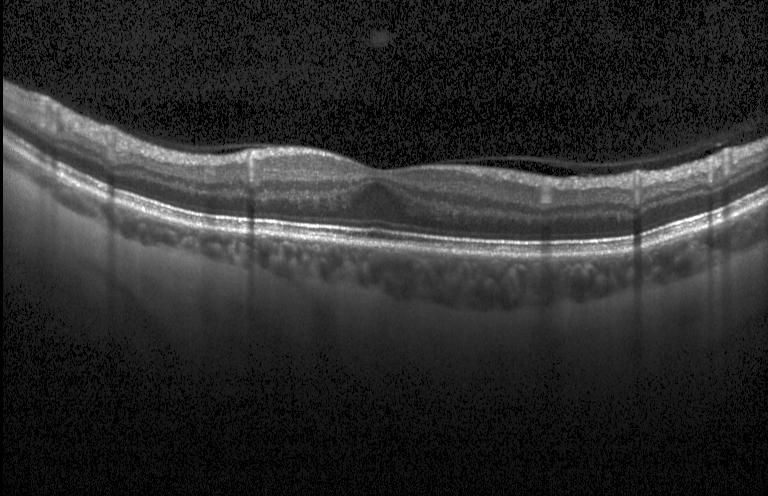

OCT line scan — Finding: neither choroidal neovascularization, diabetic macular edema, nor drusen.